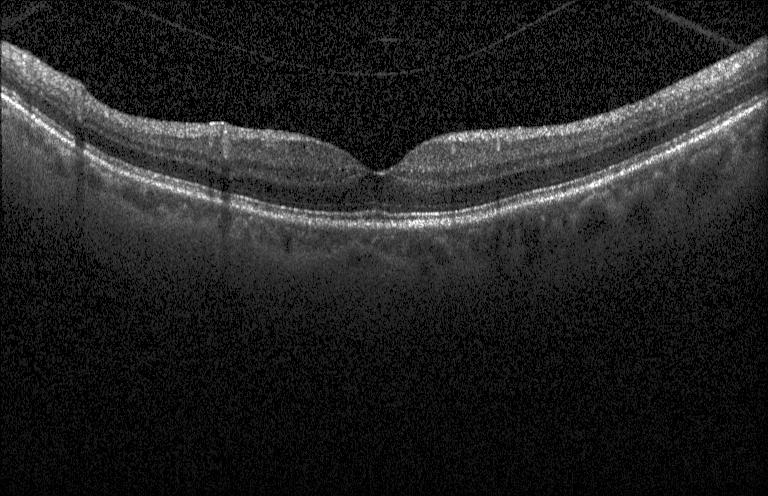 Heidelberg Spectralis · SD-OCT · optical coherence tomography scan · macular scan
Impression: no CNV, DME, or drusen.